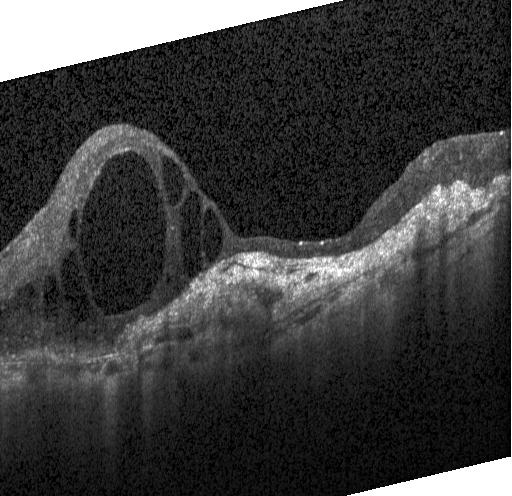
Macular OCT: choroidal neovascularization.